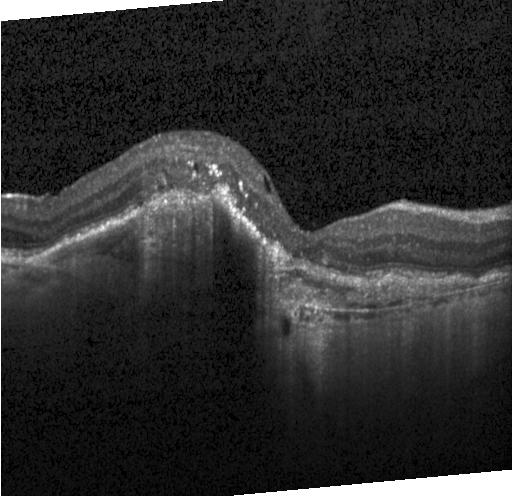

OCT B-scan.
Impression: a choroidal neovascular membrane.